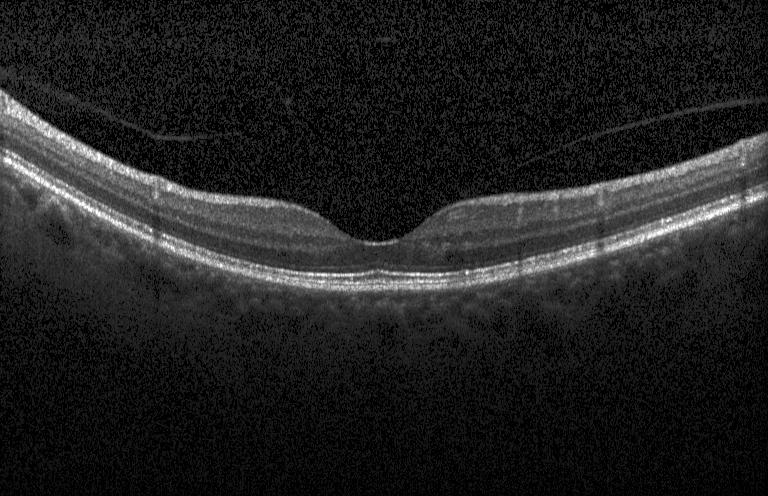 Macular OCT: neither choroidal neovascularization, diabetic macular edema, nor drusen.